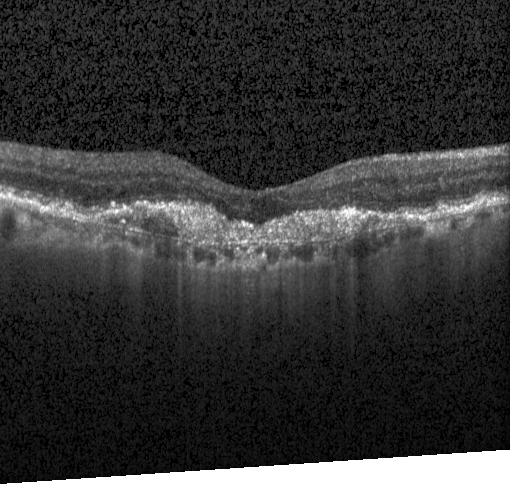 Optical coherence tomography B-scan · Heidelberg Spectralis · fovea-centered
The scan shows a choroidal neovascular membrane.